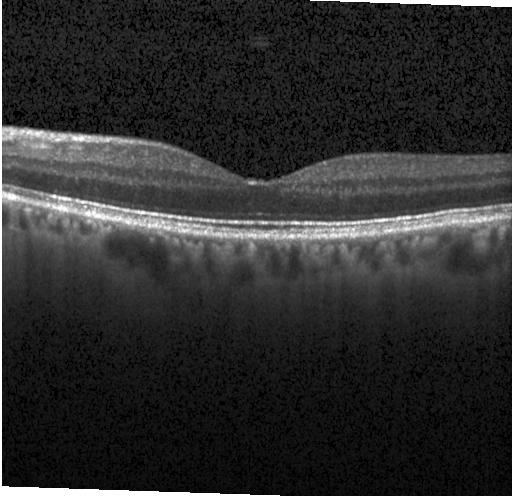 OCT B-scan; macular scan; SD-OCT — Impression: no CNV, no DME, and no drusen.